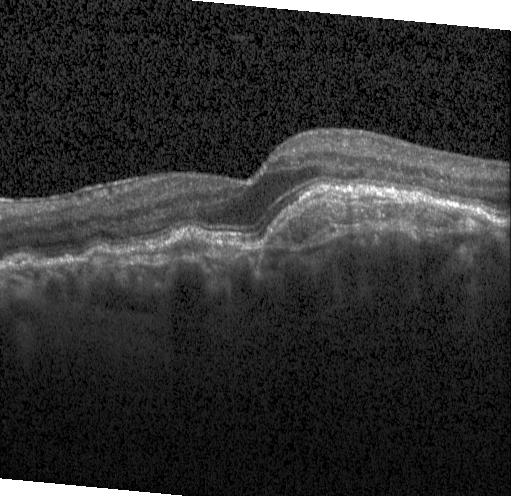 OCT B-scan showing a choroidal neovascular membrane.